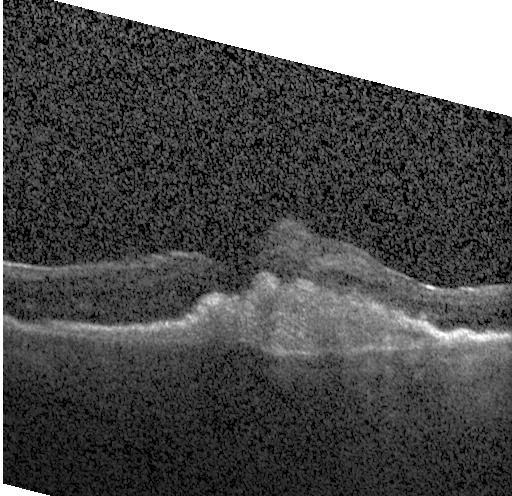

Retinal OCT cross-section
Choroidal neovascularization (CNV).